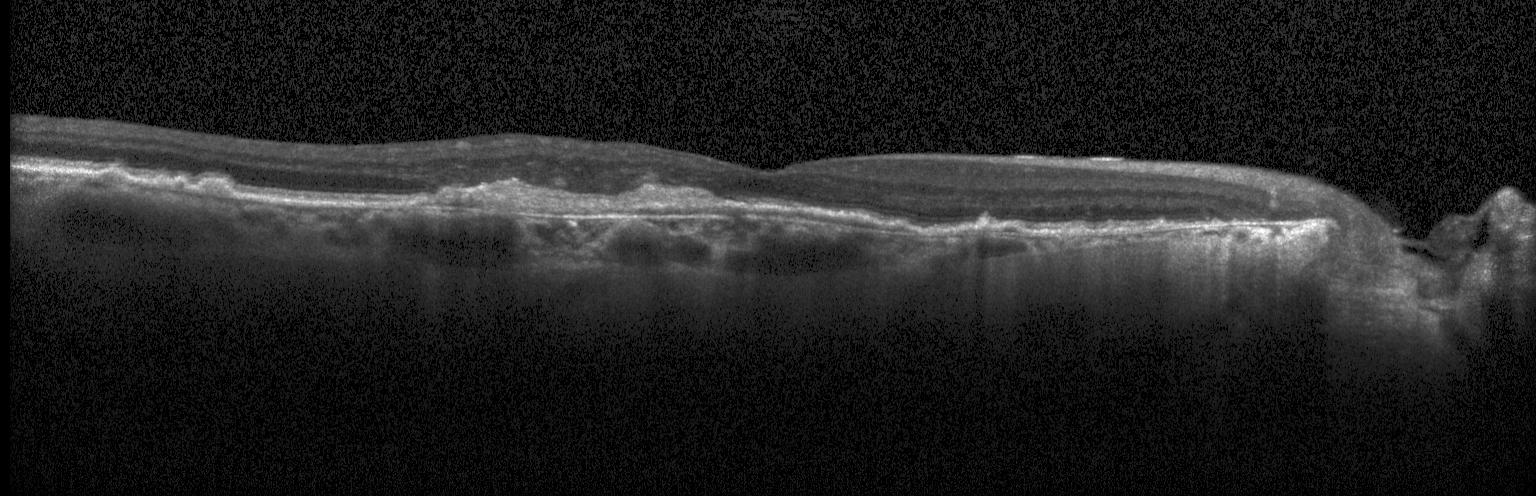
Instrument: Heidelberg Spectralis. Optical coherence tomography scan. Centered on the fovea. SD-OCT
This B-scan demonstrates choroidal neovascularization (CNV).